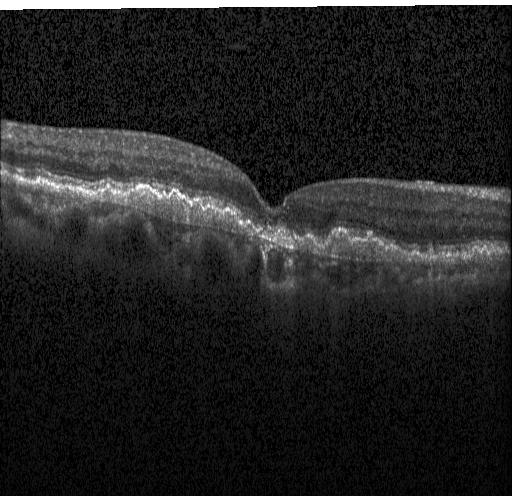 Retinal OCT cross-section.
Diagnosis: a choroidal neovascular membrane.